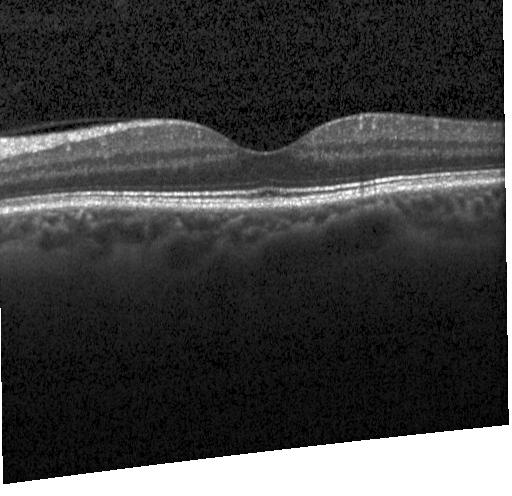
Diagnosis: no choroidal neovascularization, diabetic macular edema, or drusen.